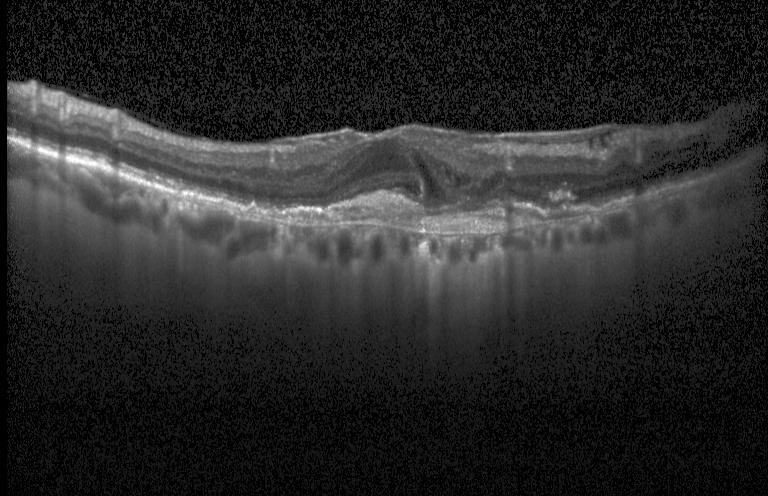 Finding: choroidal neovascularization (CNV).